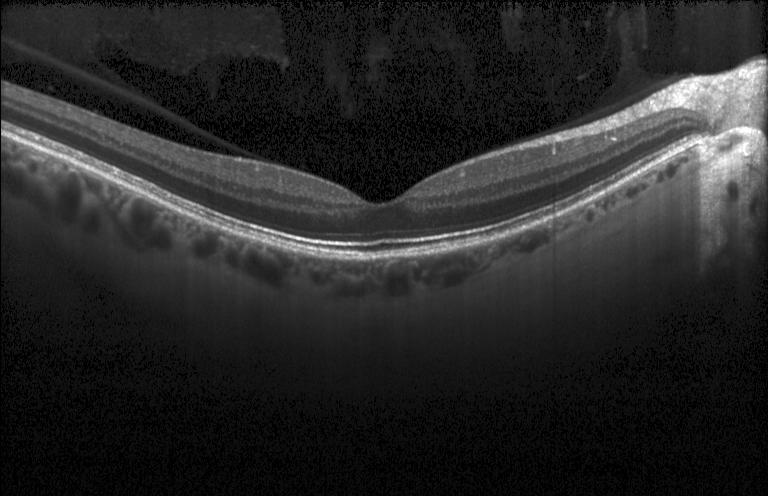 Spectral-domain optical coherence tomography, optical coherence tomography B-scan, centered on the fovea.
Neither CNV, DME, nor drusen.